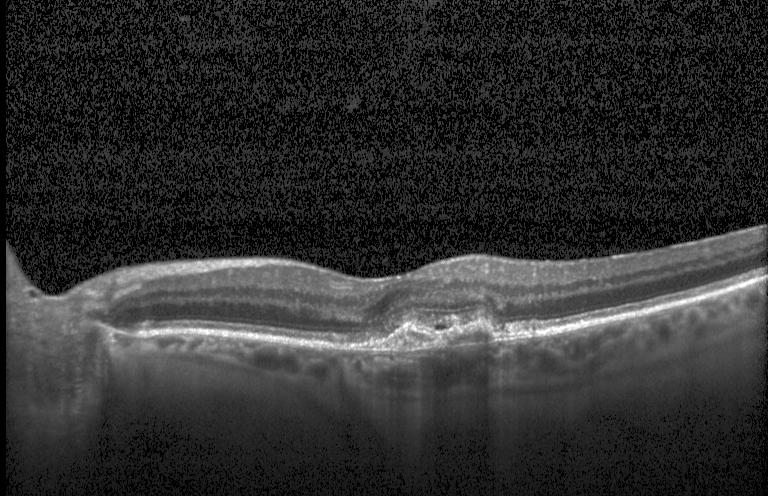

Retinal OCT B-scan. Instrument: Heidelberg Spectralis
Diagnosis: choroidal neovascularization.